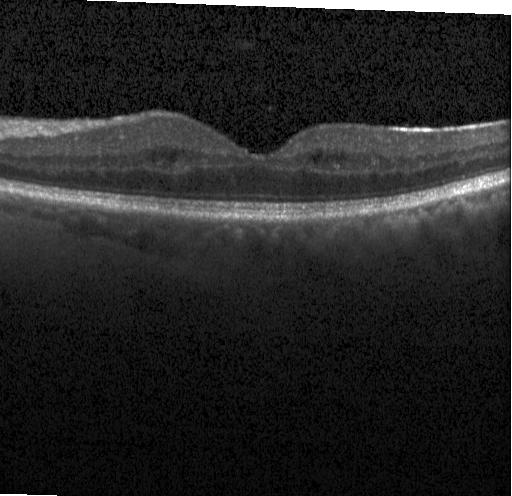 Through the macula. Retinal OCT cross-section. Heidelberg Spectralis — Finding: DME.